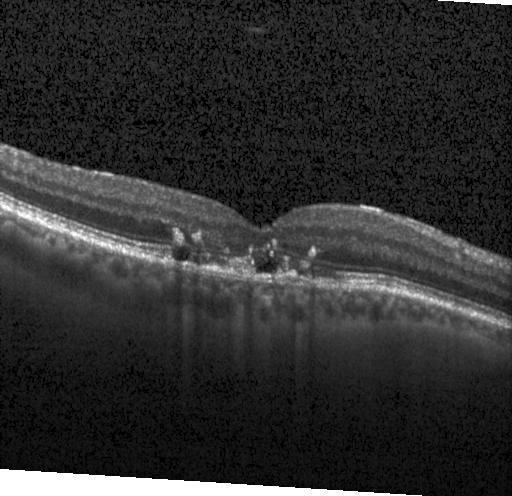 SD-OCT; Heidelberg Spectralis; optical coherence tomography scan; macular scan.
This B-scan demonstrates CNV.